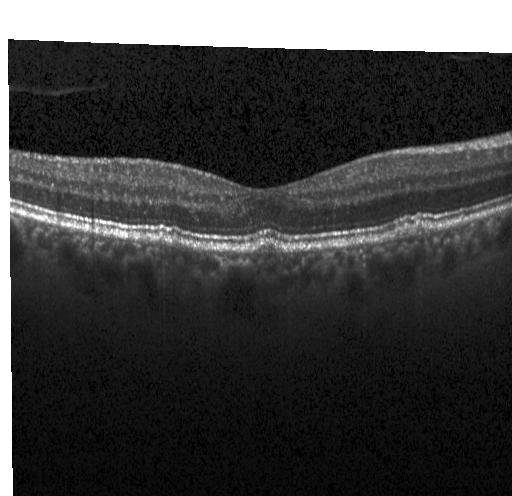

OCT finding: multiple drusen.